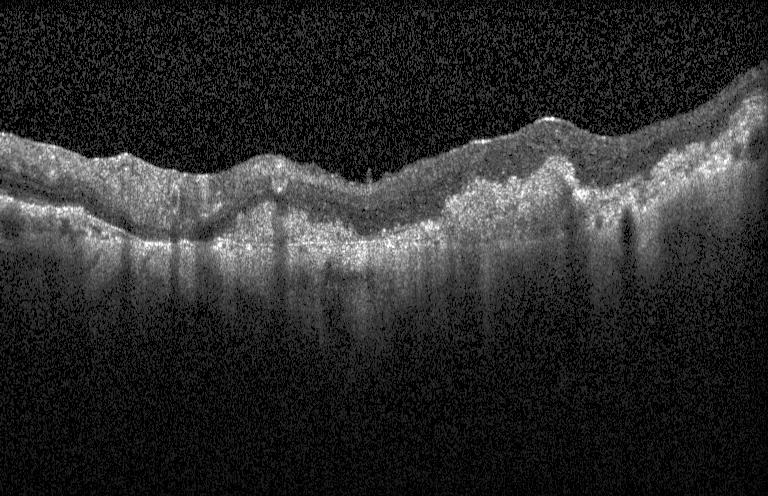 Through the macula · Heidelberg Spectralis · retinal OCT B-scan.
Diagnosis: a choroidal neovascular membrane.